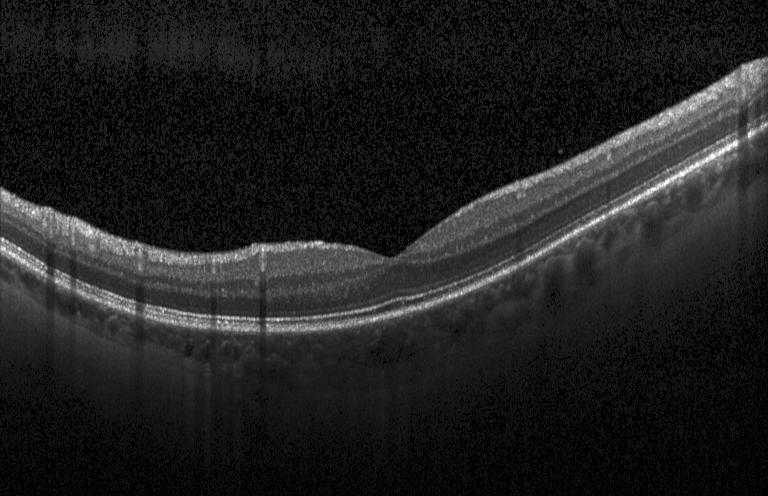

Heidelberg Spectralis OCT system. OCT B-scan
Macular OCT: neither choroidal neovascularization, diabetic macular edema, nor drusen.